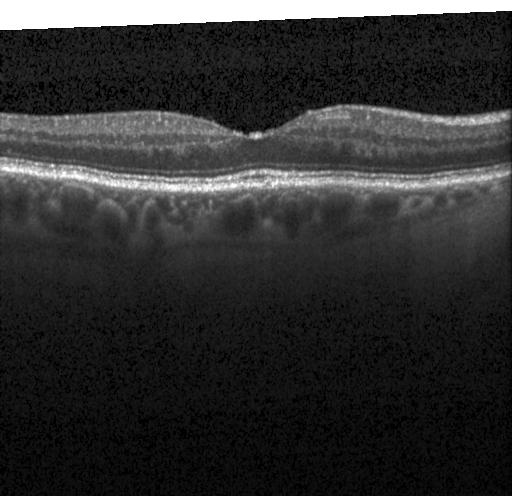 OCT scan showing no evidence of choroidal neovascularization, diabetic macular edema, or drusen.